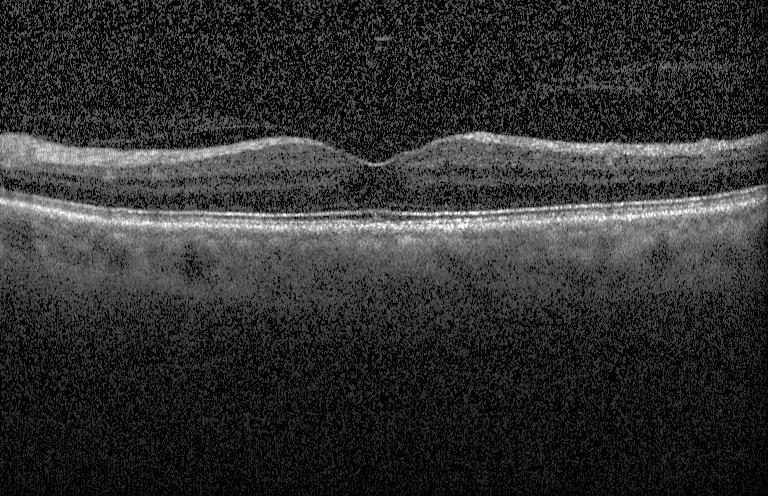
Retinal OCT cross-section. Assessment: neither choroidal neovascularization, diabetic macular edema, nor drusen.